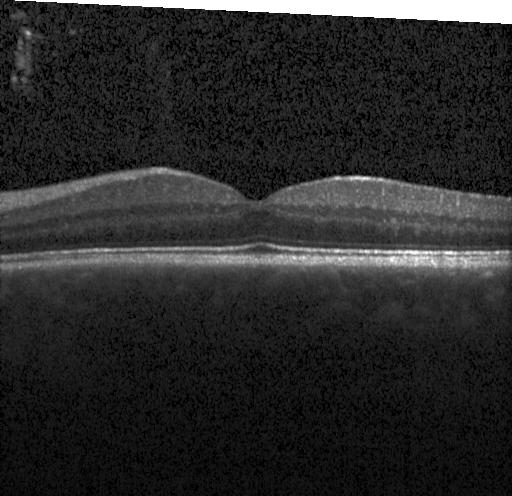

Finding: neither CNV, DME, nor drusen.